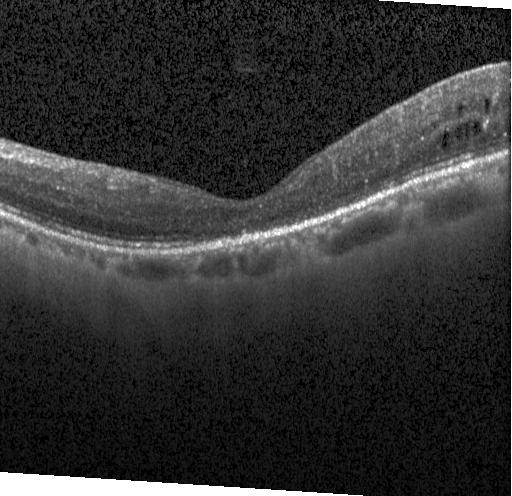
Macular OCT: diabetic macular edema (DME).